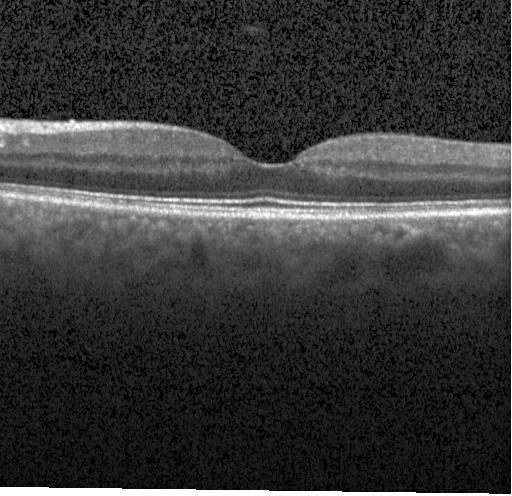
Dx: neither choroidal neovascularization, diabetic macular edema, nor drusen.